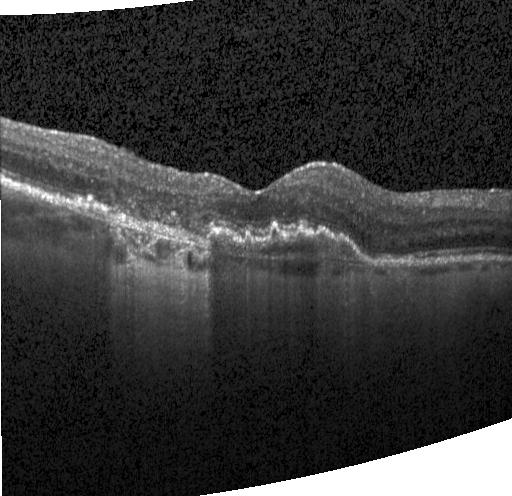

Diagnosis: CNV.